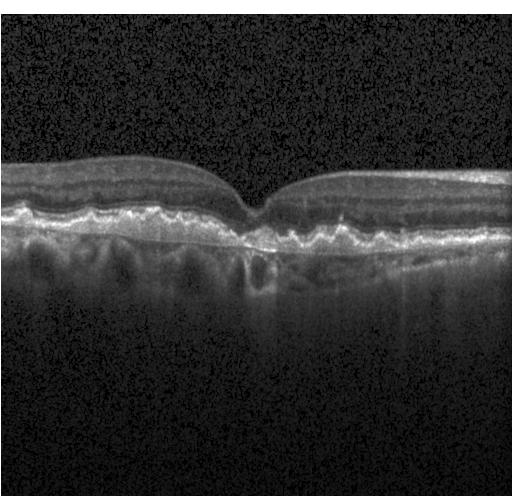
Optical coherence tomography scan, fovea-centered.
Diagnosis: a choroidal neovascular membrane.